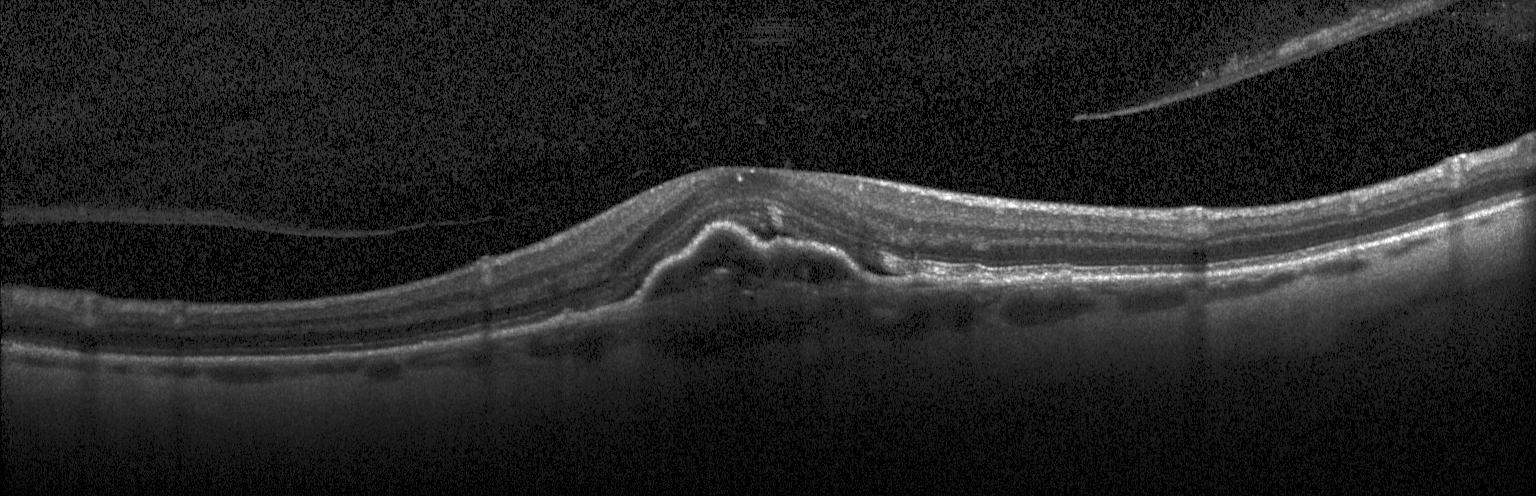 Macular OCT: choroidal neovascularization (CNV).